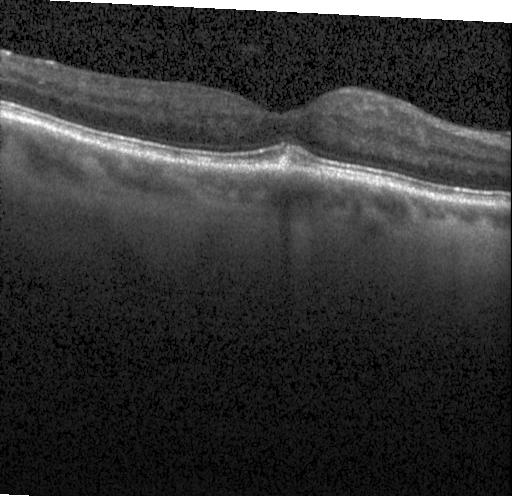
Finding: multiple drusen.